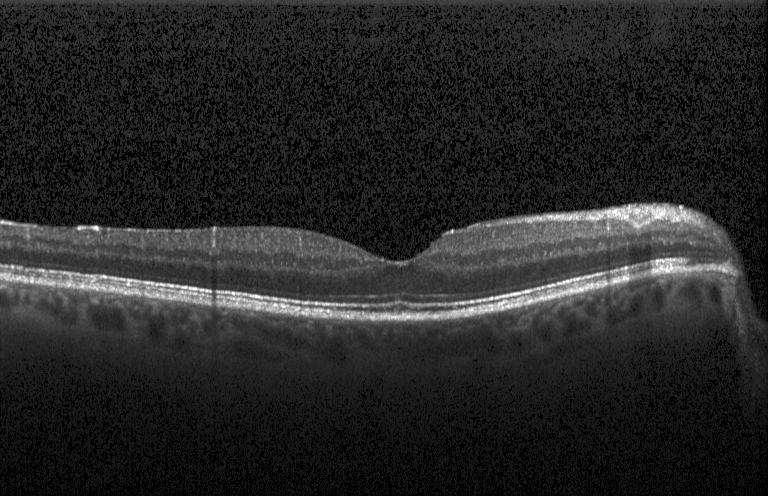 OCT B-scan showing no CNV, DME, or drusen.